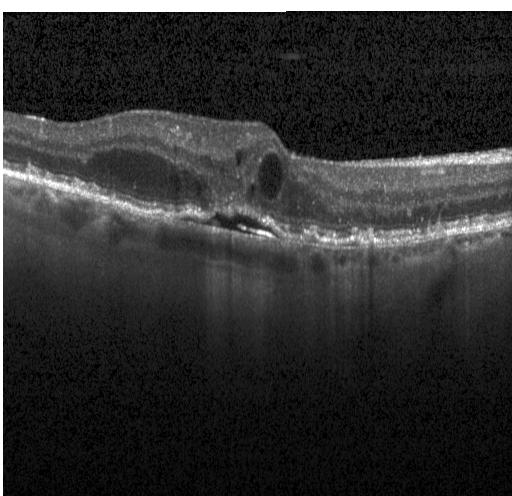

Retinal OCT cross-section
OCT finding: choroidal neovascularization.